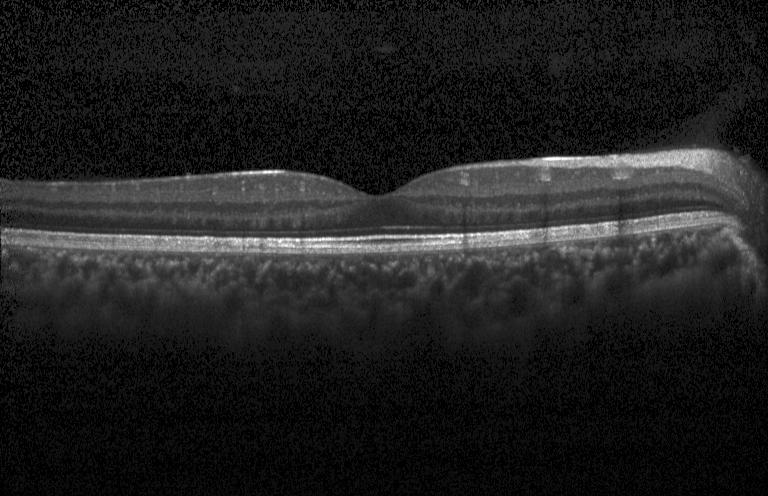

Spectral-domain optical coherence tomography; optical coherence tomography scan; horizontal scan through the fovea — Diagnosis: no choroidal neovascularization, diabetic macular edema, or drusen.